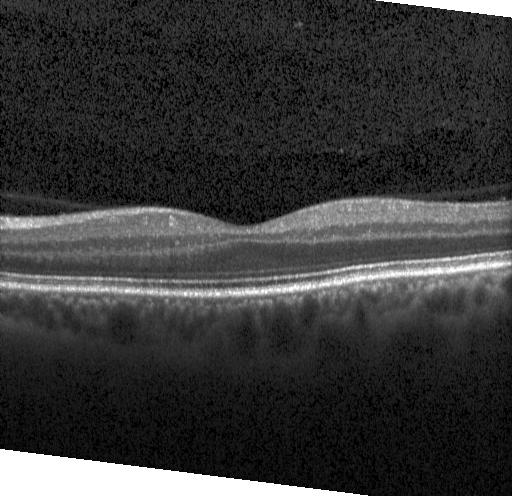
Centered on the fovea, optical coherence tomography scan, Heidelberg Spectralis OCT system
OCT finding: no CNV, DME, or drusen.